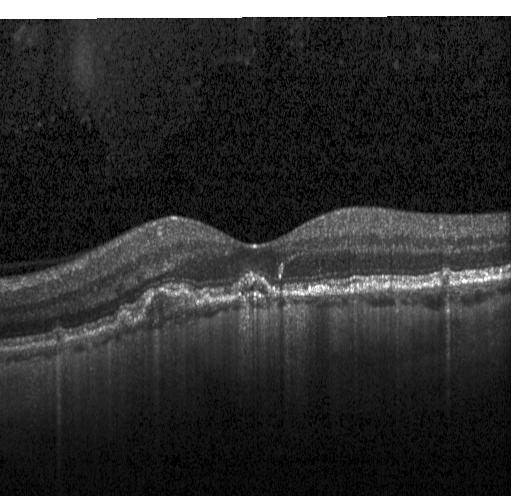

Optical coherence tomography B-scan. Finding: CNV.